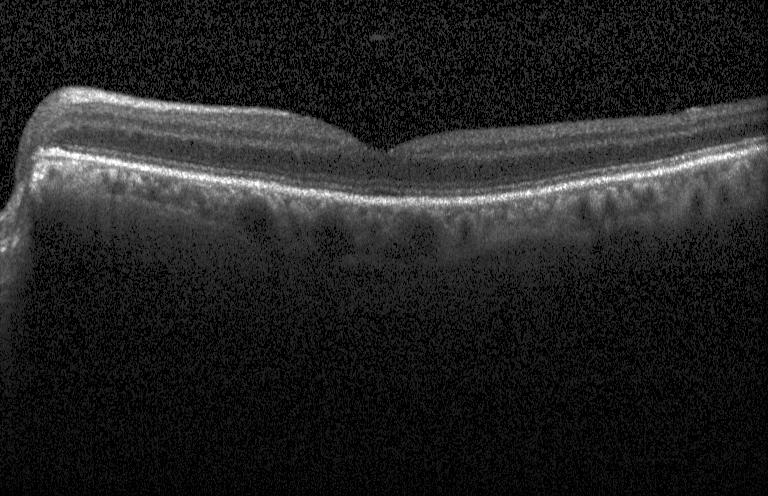
Spectral-domain OCT B-scan: no evidence of choroidal neovascularization, diabetic macular edema, or drusen.